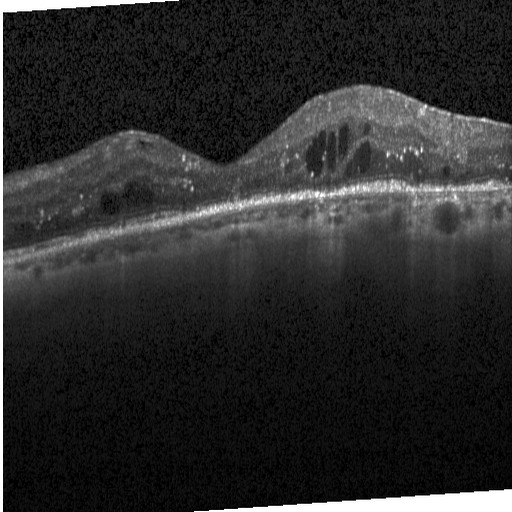
Dx: diabetic macular edema.